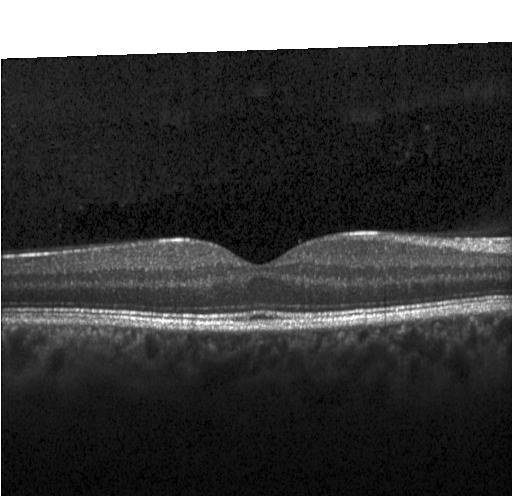
Spectral-domain OCT. OCT line scan
Assessment: no choroidal neovascularization, no diabetic macular edema, and no drusen.